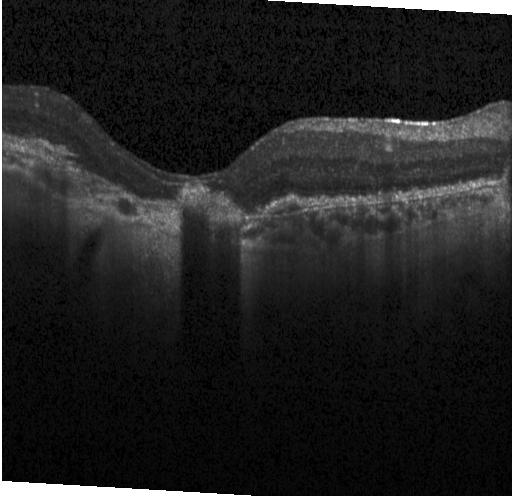
A choroidal neovascular membrane.